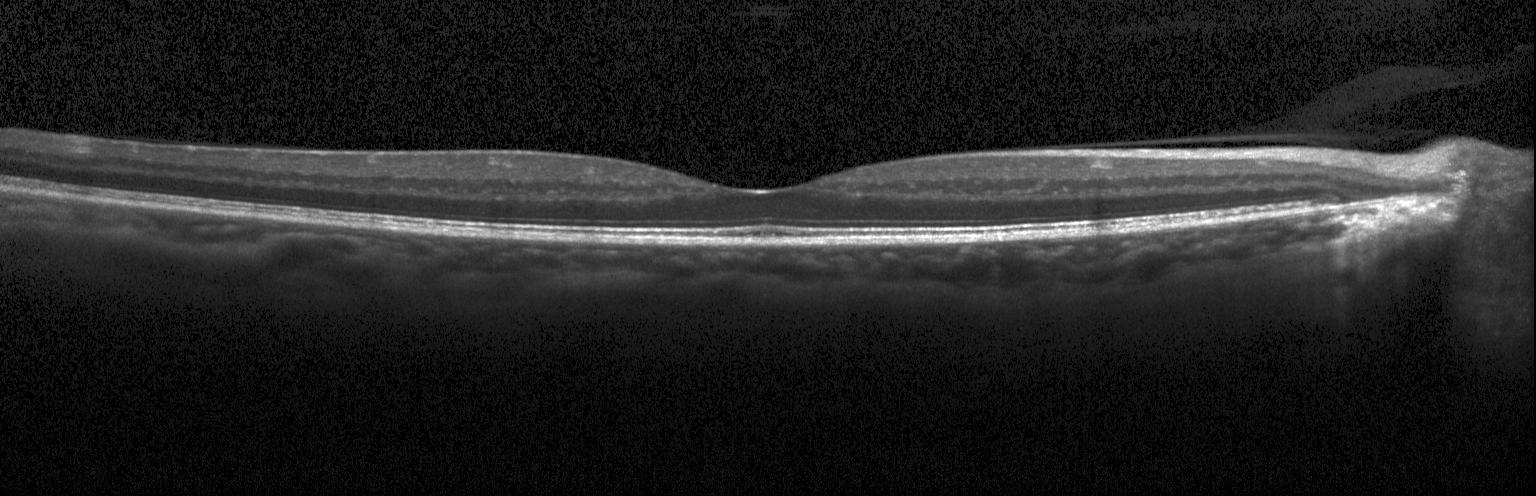

The scan shows no choroidal neovascularization, diabetic macular edema, or drusen.